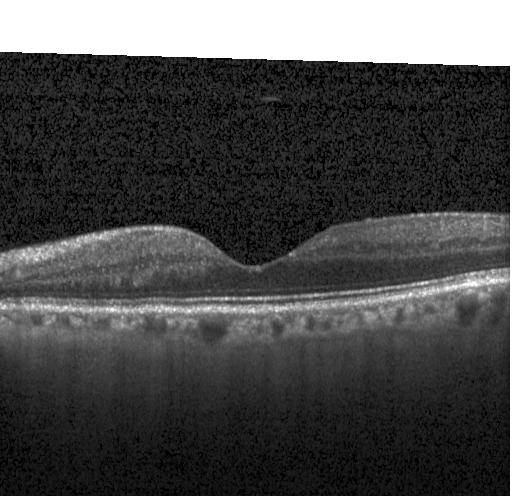 Fovea-centered · SD-OCT · retinal OCT B-scan.
Assessment: no choroidal neovascularization, diabetic macular edema, or drusen.